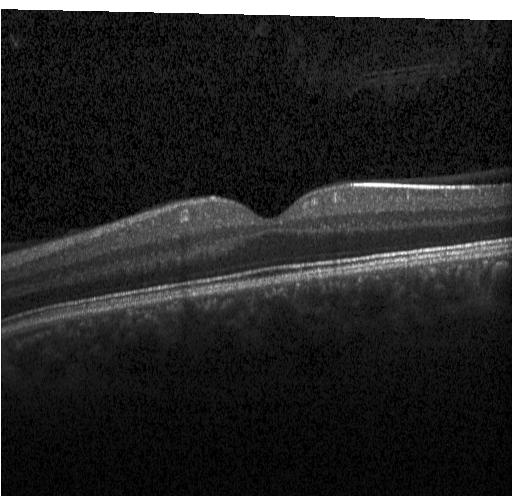

Dx: no choroidal neovascularization, no diabetic macular edema, and no drusen.